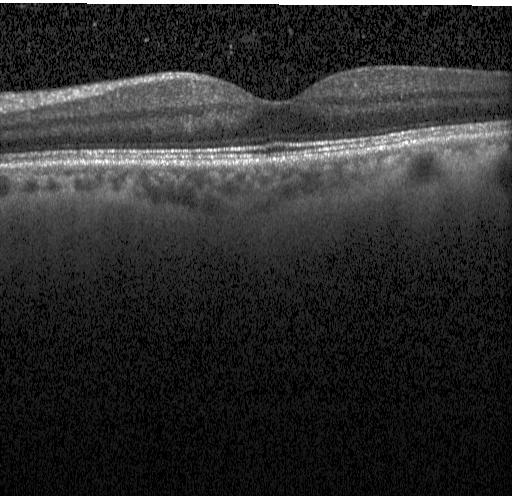

OCT B-scan · acquired on a Heidelberg Spectralis — Impression: no evidence of choroidal neovascularization, diabetic macular edema, or drusen.